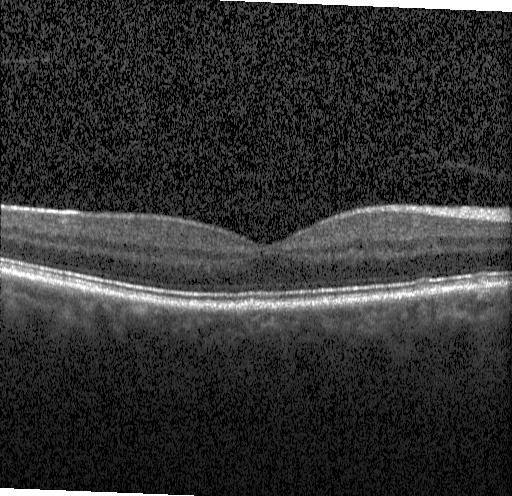
Heidelberg Spectralis OCT system · retinal OCT B-scan — No choroidal neovascularization, diabetic macular edema, or drusen.